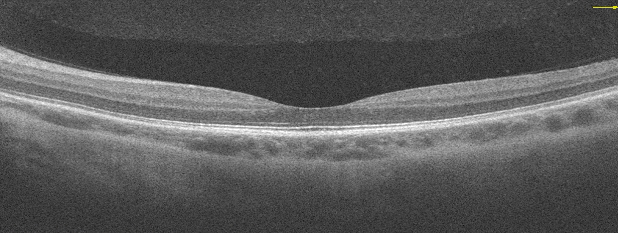
Through the macula. Optovue Avanti RTVue XR. Optical coherence tomography B-scan. Assessment: no evidence of AMD, DME, ERM, RAO, RVO, or VID.